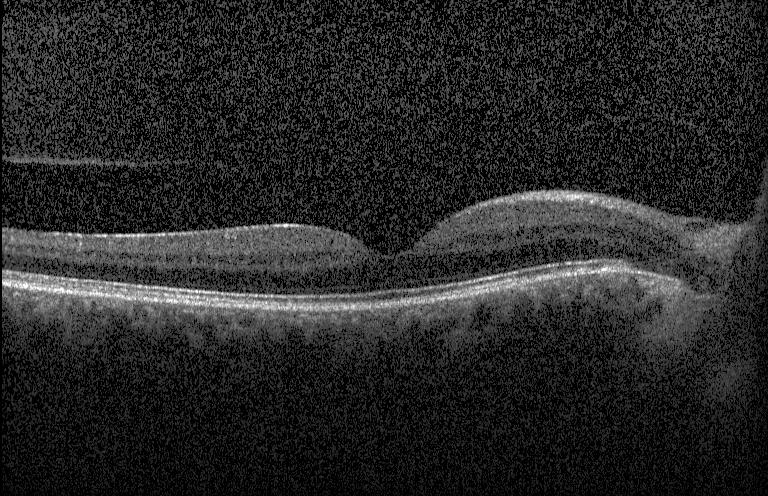 The scan shows neither CNV, DME, nor drusen.